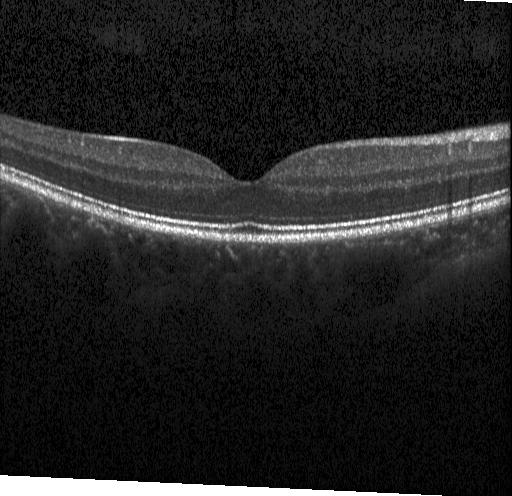

Macular OCT: no CNV, DME, or drusen.